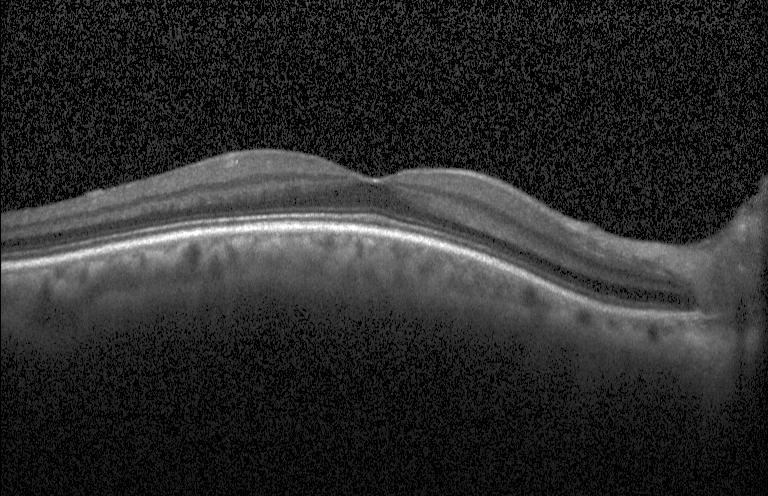
Macular scan · spectral-domain optical coherence tomography · optical coherence tomography B-scan · Heidelberg Spectralis. Diagnosis: no evidence of choroidal neovascularization, diabetic macular edema, or drusen.